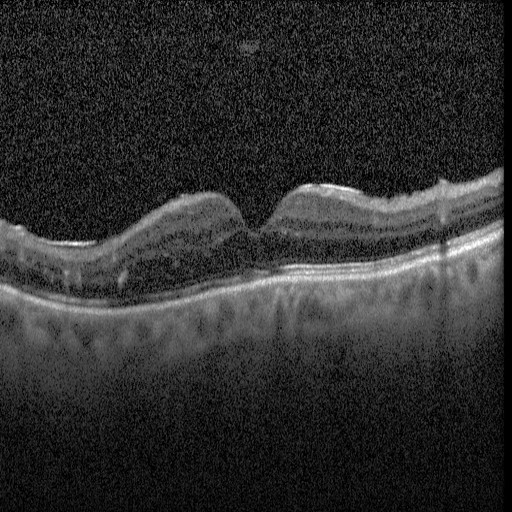 OCT line scan
Finding: diabetic macular edema (DME).